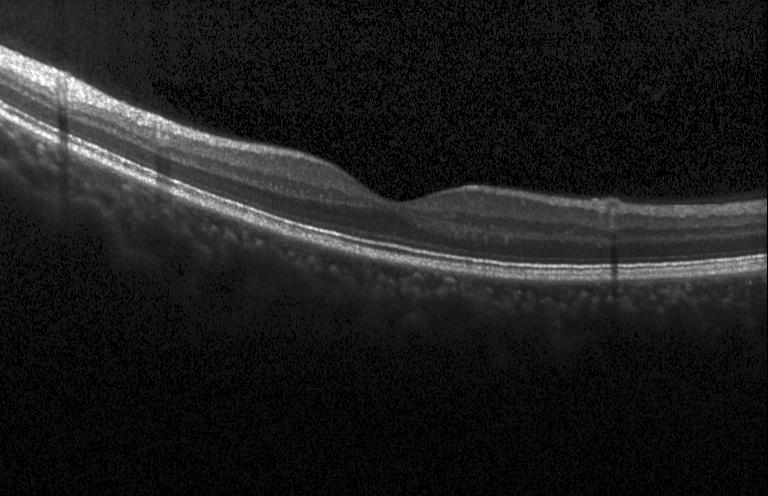
Macular scan; Heidelberg Spectralis OCT system; OCT B-scan; spectral-domain optical coherence tomography.
Impression: no CNV, DME, or drusen.